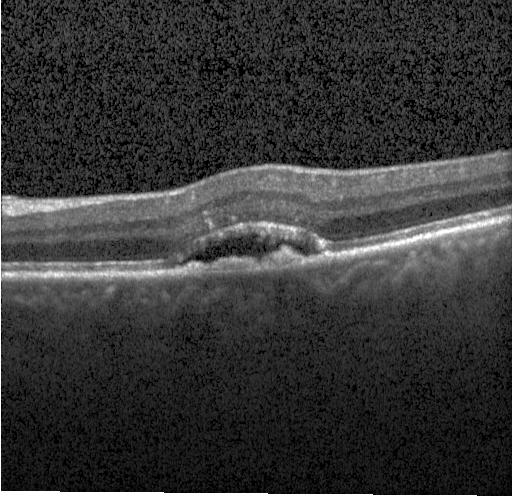
Spectral-domain OCT · optical coherence tomography scan · centered on the fovea. Dx: a choroidal neovascular membrane.